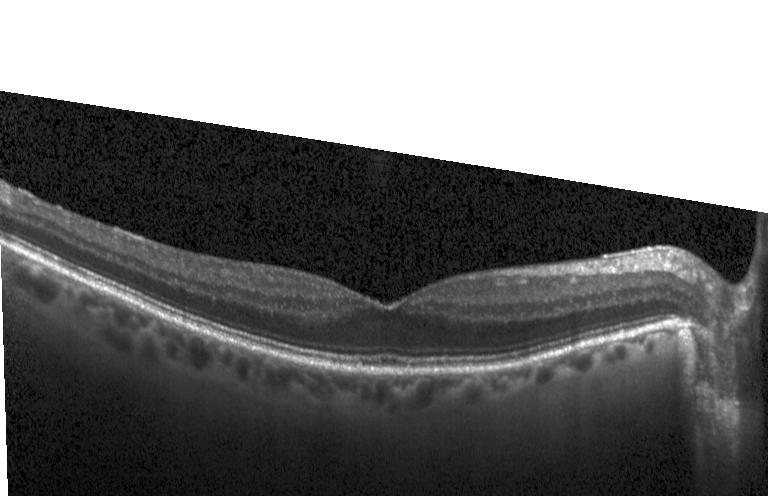

Spectral-domain OCT. OCT line scan. Macular scan — This B-scan demonstrates no evidence of choroidal neovascularization, diabetic macular edema, or drusen.